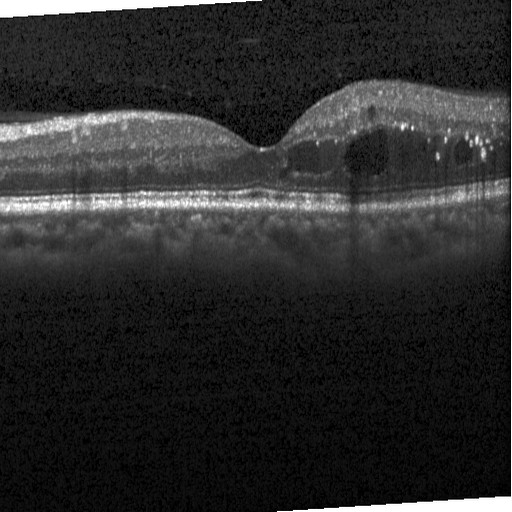
Impression: DME.